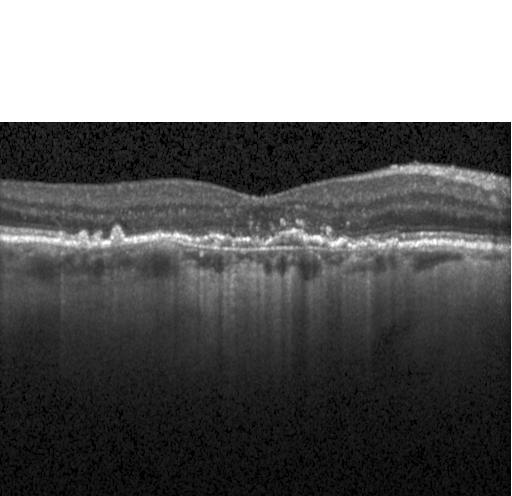 SD-OCT; retinal OCT B-scan. Diagnosis: choroidal neovascularization (CNV).